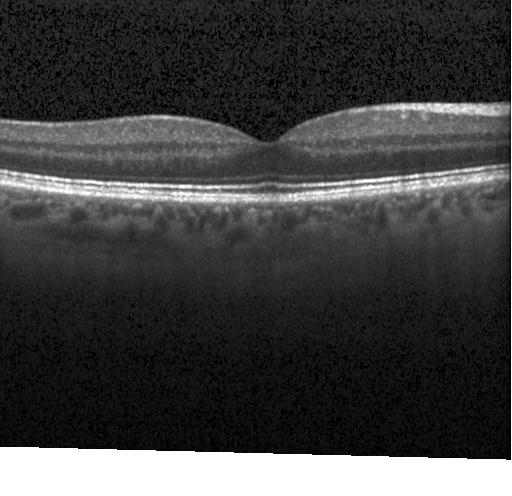
Fovea-centered, retinal OCT cross-section
Assessment: no choroidal neovascularization, diabetic macular edema, or drusen.